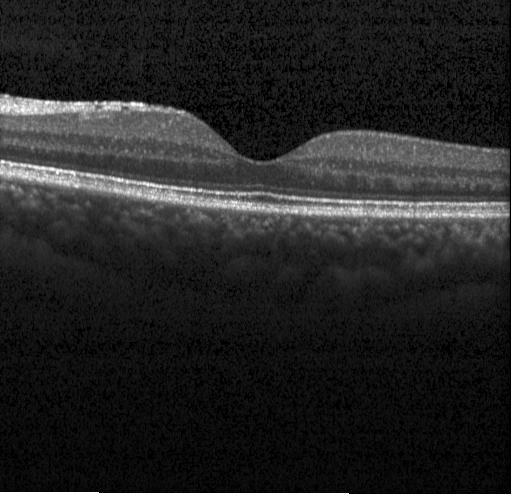 Diagnosis: no evidence of choroidal neovascularization, diabetic macular edema, or drusen.